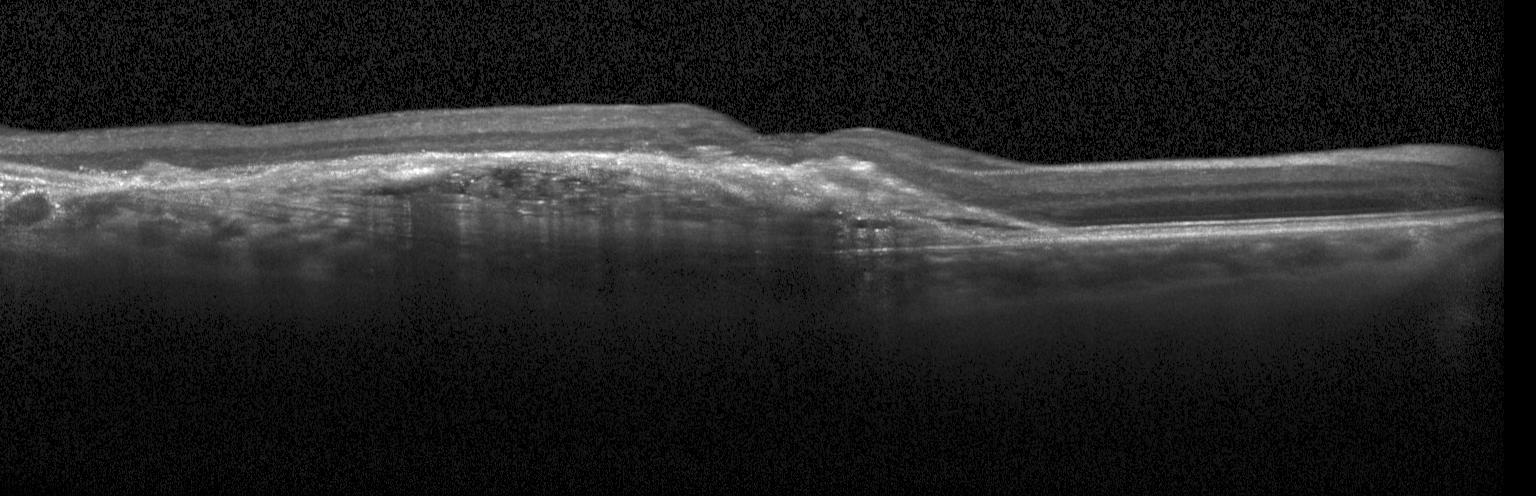 Finding: choroidal neovascularization (CNV).